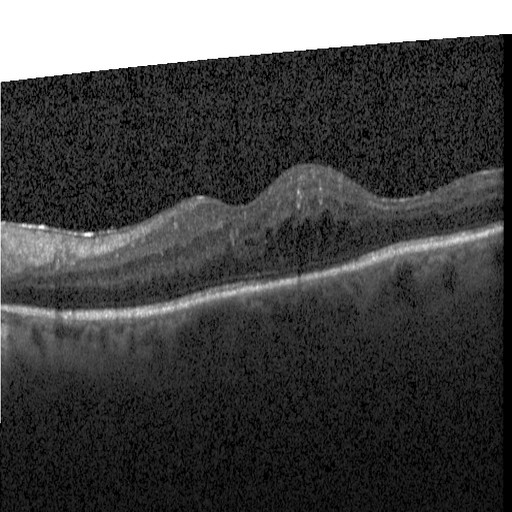

Assessment: DME.